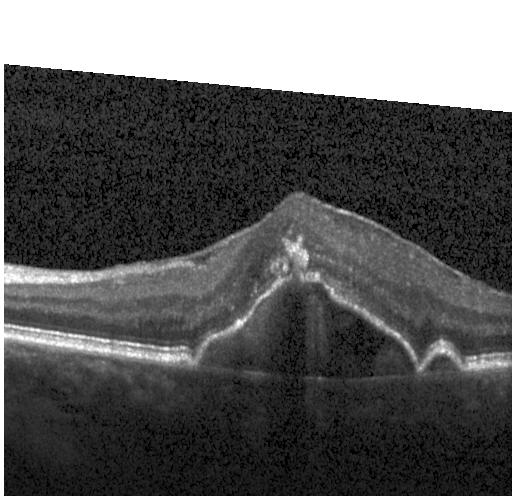

Retinal OCT cross-section — Finding: a choroidal neovascular membrane.